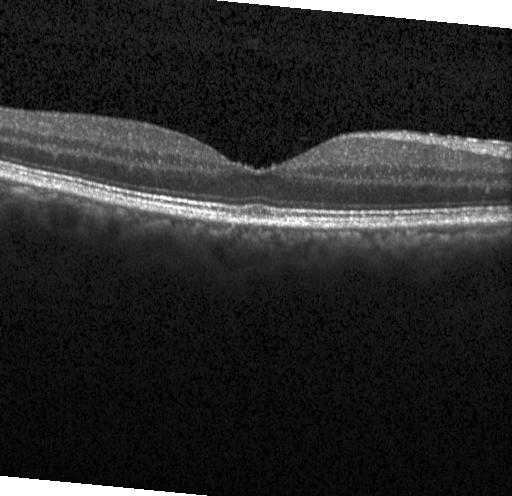
Heidelberg Spectralis; retinal OCT B-scan.
Finding: no evidence of choroidal neovascularization, diabetic macular edema, or drusen.